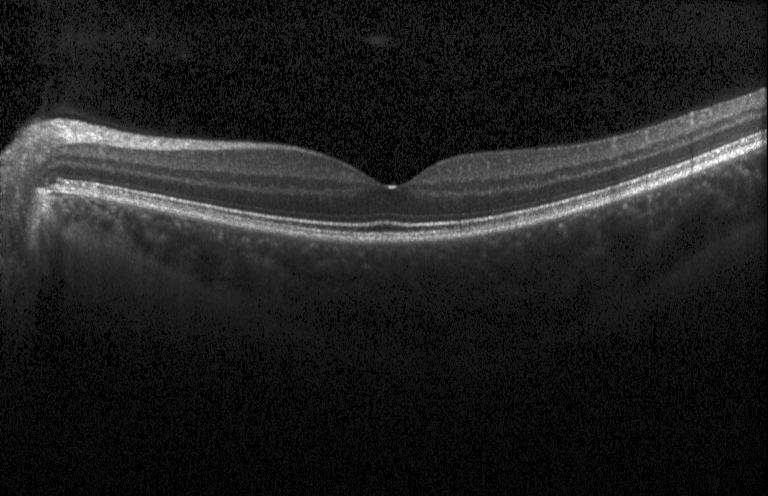
Assessment: neither choroidal neovascularization, diabetic macular edema, nor drusen.